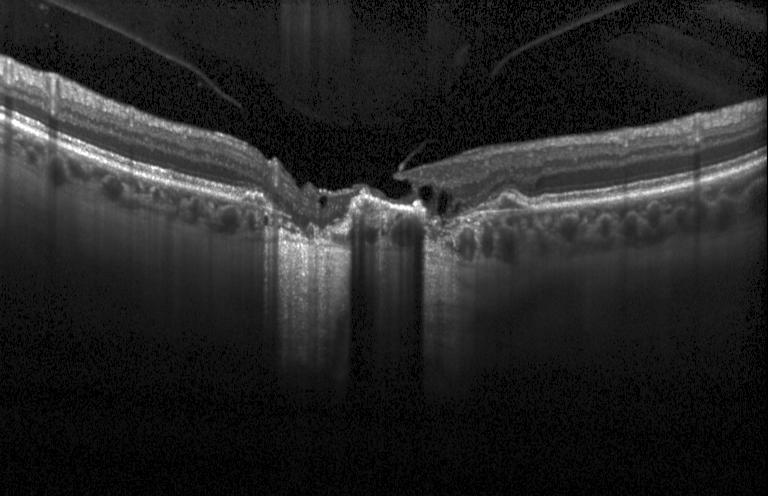 Spectral-domain optical coherence tomography, retinal OCT cross-section
Assessment: a choroidal neovascular membrane.